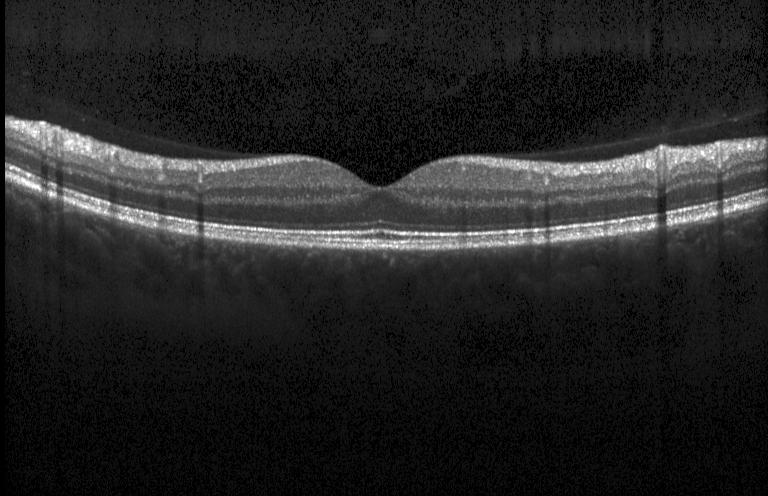

Spectral-domain OCT, Heidelberg Spectralis OCT system, OCT B-scan, fovea-centered
Diagnosis: no evidence of CNV, DME, or drusen.